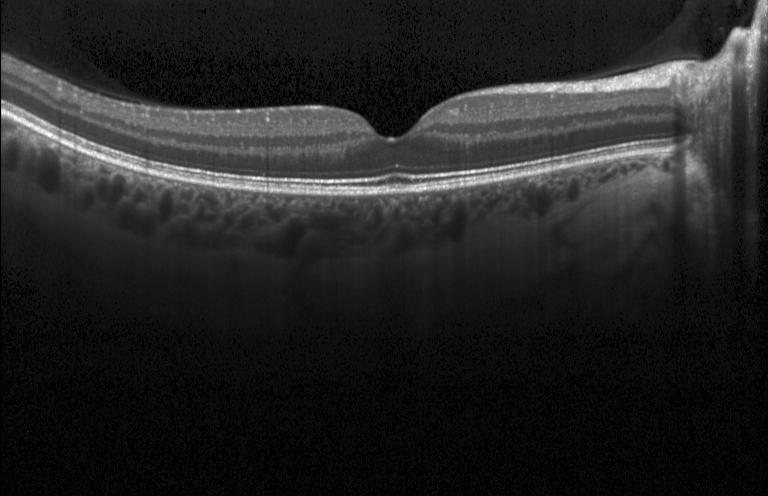

Spectral-domain optical coherence tomography, retinal OCT B-scan, Heidelberg Spectralis.
The scan shows no evidence of choroidal neovascularization, diabetic macular edema, or drusen.